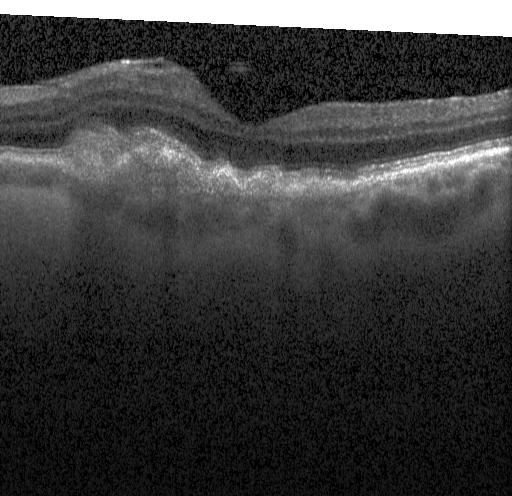 Spectral-domain OCT; instrument: Heidelberg Spectralis; OCT B-scan; macular scan.
Assessment: choroidal neovascularization.